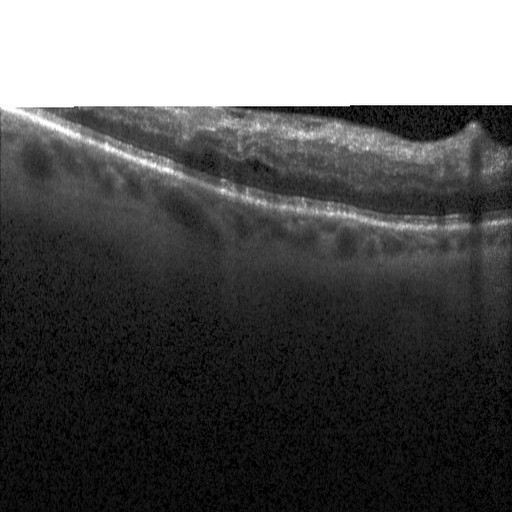

Retinal OCT cross-section — Diabetic macular edema.